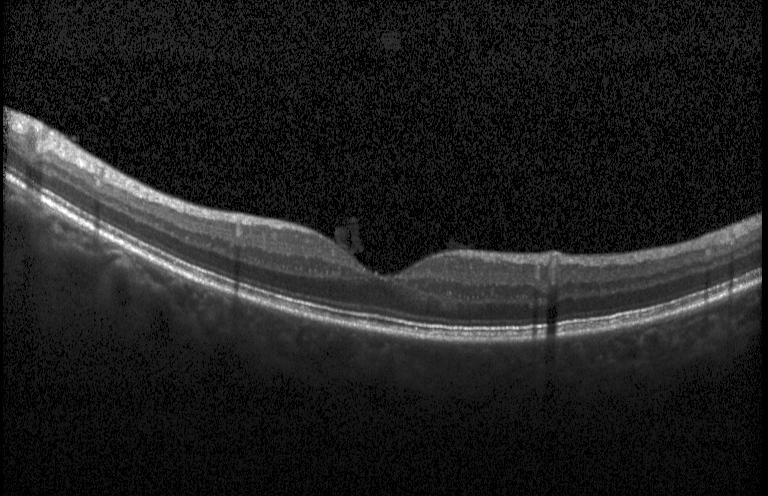

OCT line scan; SD-OCT.
No choroidal neovascularization, no diabetic macular edema, and no drusen.